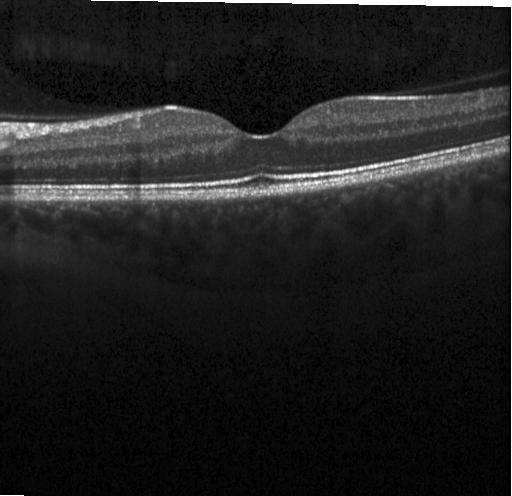 Through the macula; retinal OCT B-scan; instrument: Heidelberg Spectralis.
Macular OCT: neither choroidal neovascularization, diabetic macular edema, nor drusen.